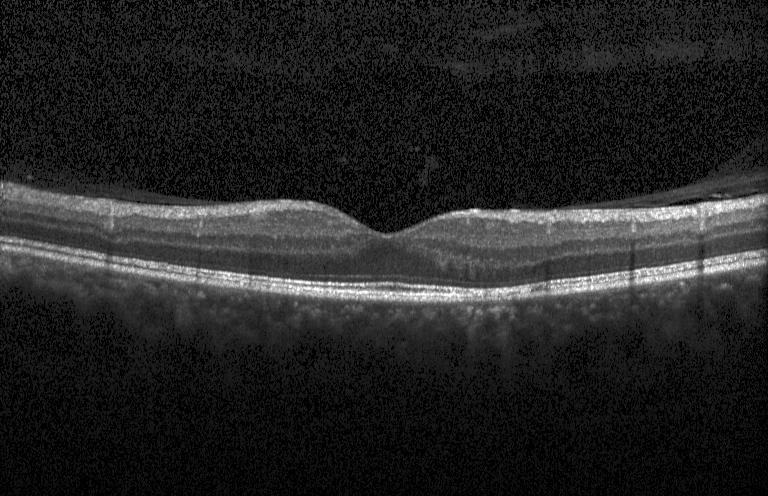
OCT B-scan. Assessment: no choroidal neovascularization, no diabetic macular edema, and no drusen.